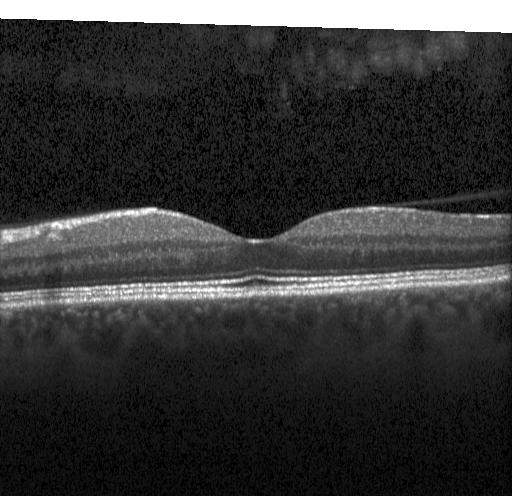
This B-scan demonstrates no choroidal neovascularization, no diabetic macular edema, and no drusen.